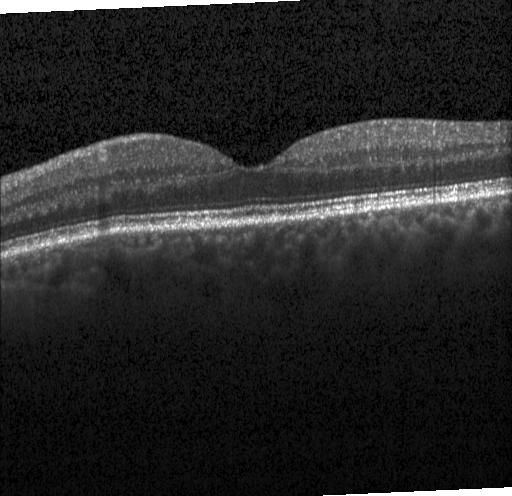

This B-scan demonstrates no evidence of choroidal neovascularization, diabetic macular edema, or drusen.